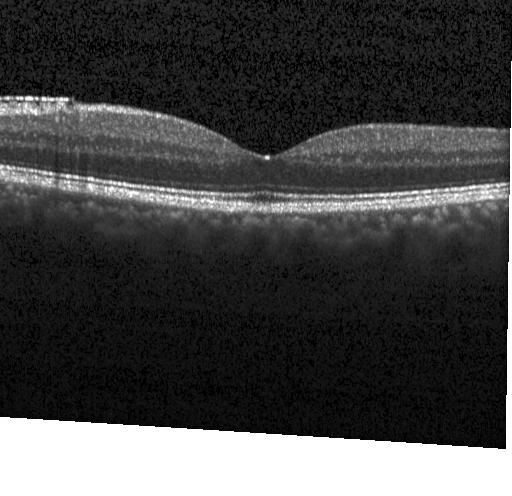
OCT B-scan · horizontal scan through the fovea · SD-OCT
Finding: no choroidal neovascularization, diabetic macular edema, or drusen.